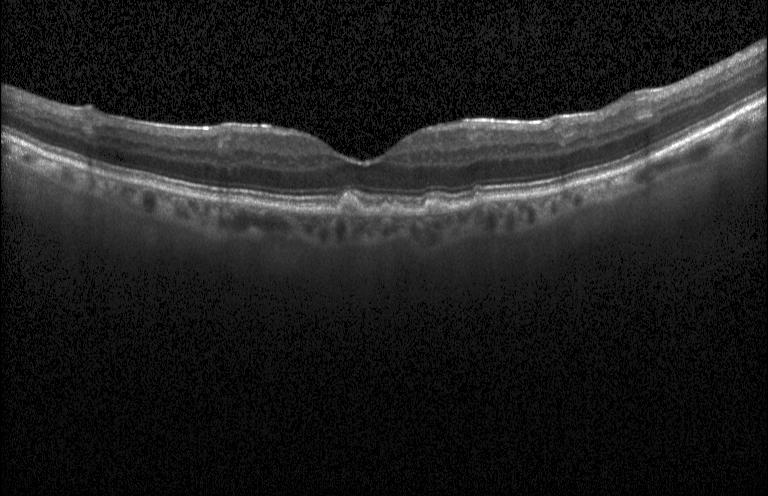
OCT B-scan showing sub-RPE drusenoid deposits.